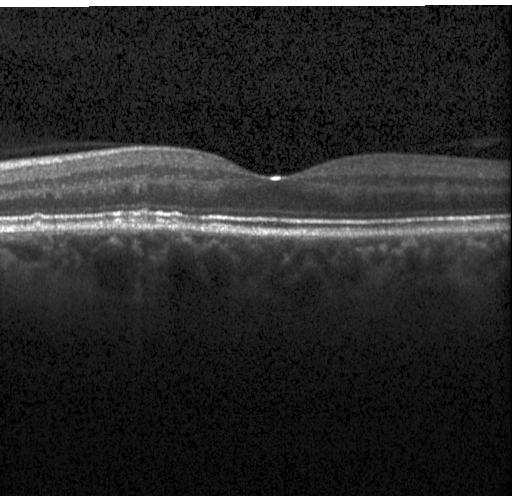
OCT B-scan showing sub-RPE drusenoid deposits.